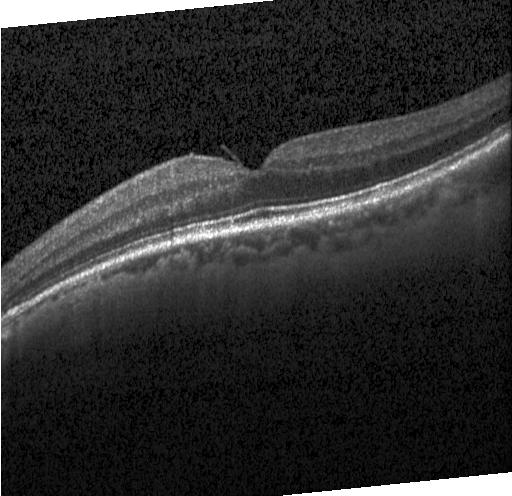

Finding: no evidence of choroidal neovascularization, diabetic macular edema, or drusen.